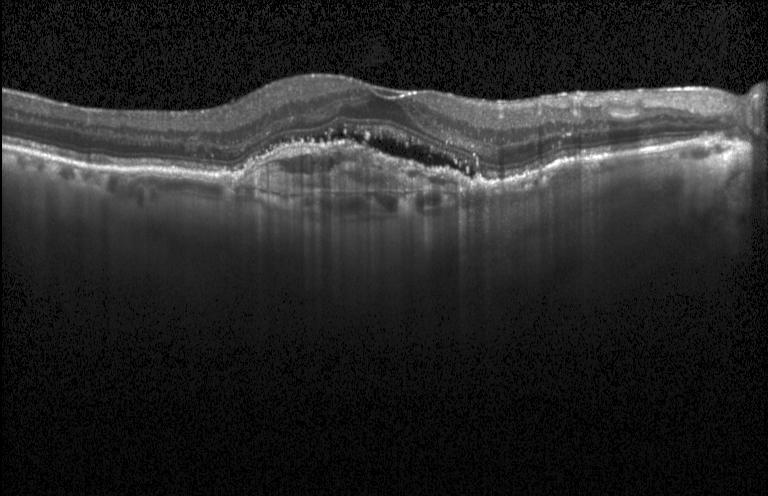
Spectral-domain optical coherence tomography, retinal OCT cross-section, Heidelberg Spectralis OCT system, centered on the fovea. Assessment: CNV.